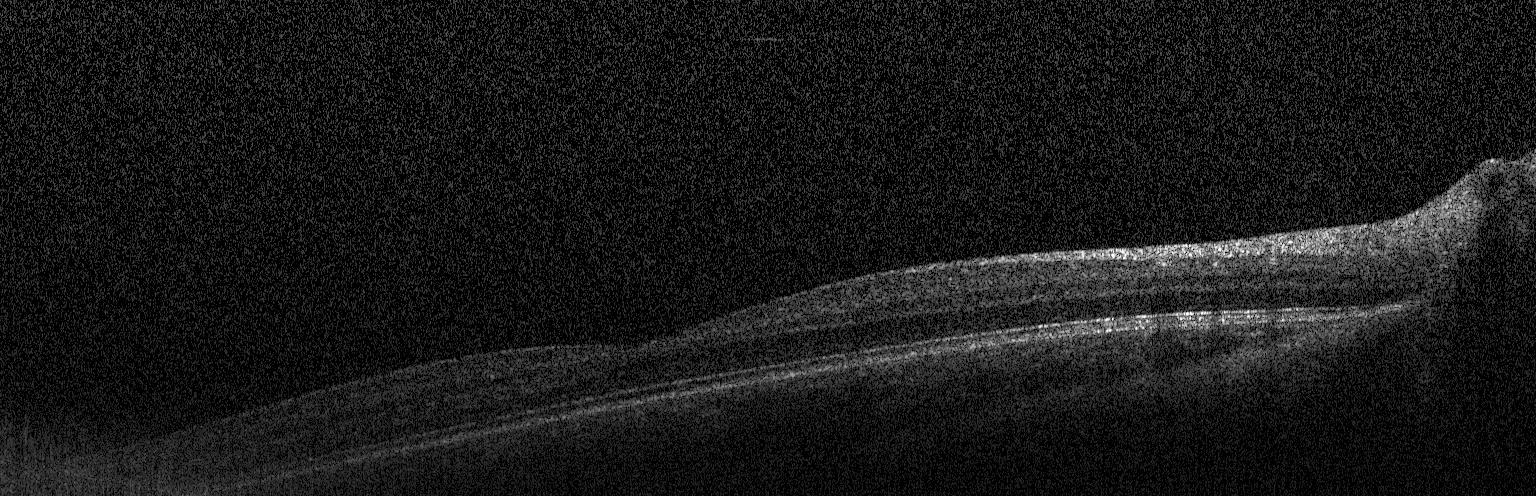
Optical coherence tomography scan. Impression: no choroidal neovascularization, no diabetic macular edema, and no drusen.